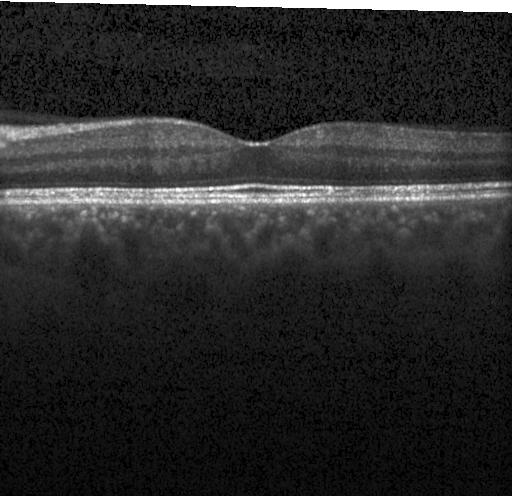 OCT finding: neither CNV, DME, nor drusen.